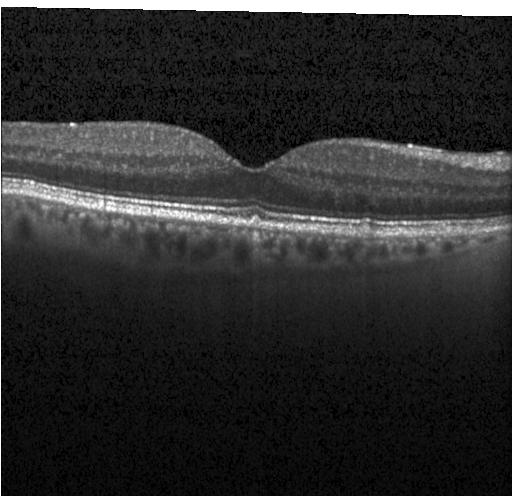 Spectral-domain optical coherence tomography; OCT B-scan. The scan shows drusen.